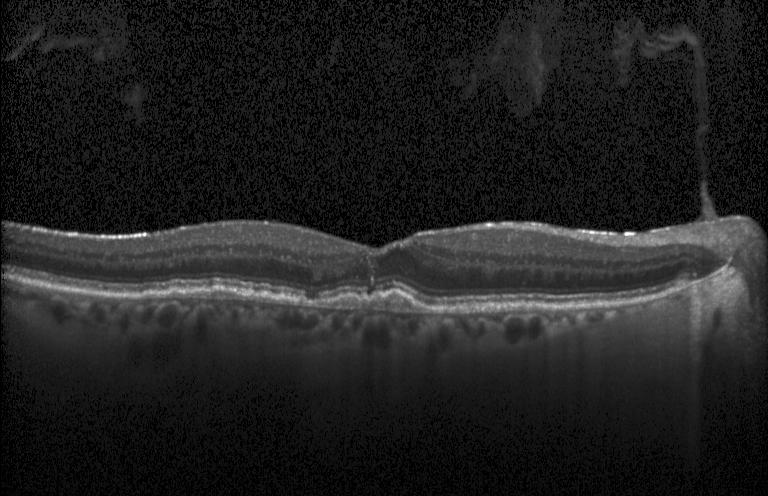

SD-OCT, optical coherence tomography scan
Diagnosis: a choroidal neovascular membrane.